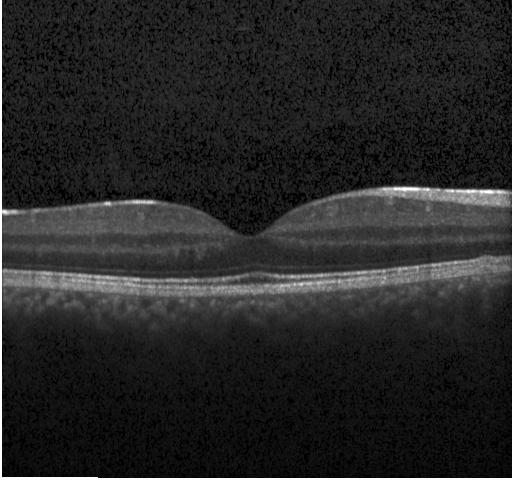
Acquired on a Heidelberg Spectralis, OCT B-scan, spectral-domain optical coherence tomography
Diagnosis: no evidence of choroidal neovascularization, diabetic macular edema, or drusen.